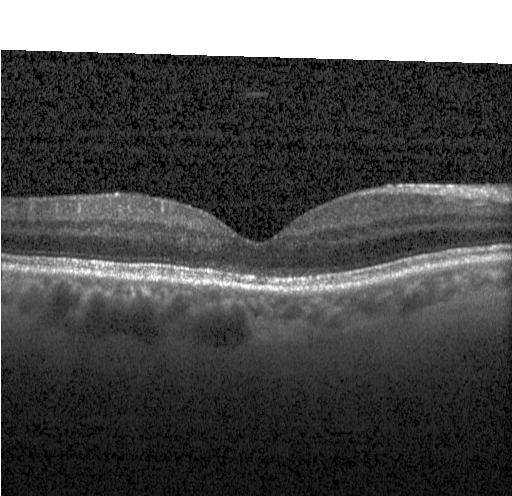 Diagnosis: no choroidal neovascularization, diabetic macular edema, or drusen.